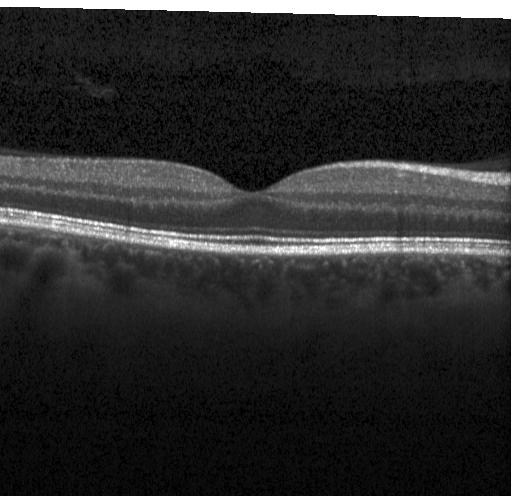

Impression: no evidence of choroidal neovascularization, diabetic macular edema, or drusen.